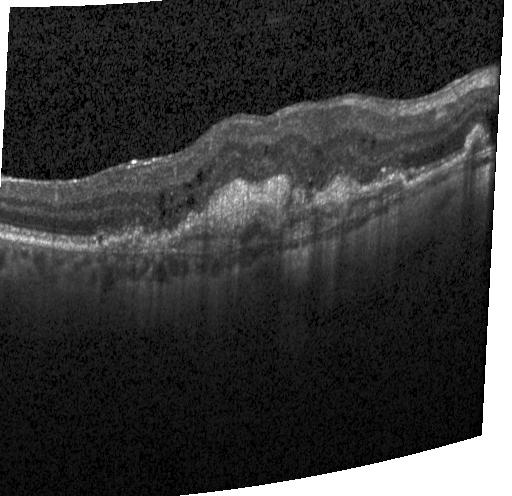
Through the macula. Spectral-domain OCT. Optical coherence tomography B-scan. This B-scan demonstrates a choroidal neovascular membrane.